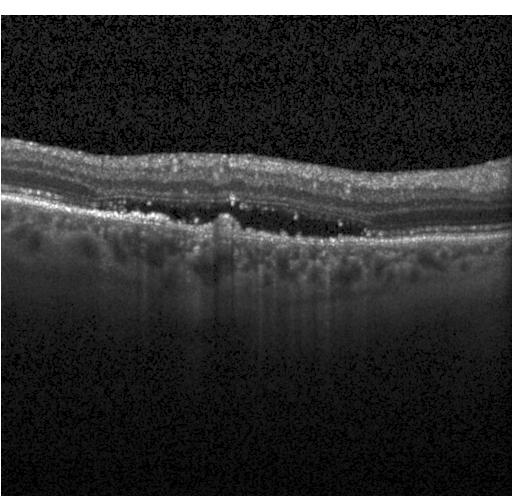

Diagnosis: a choroidal neovascular membrane.